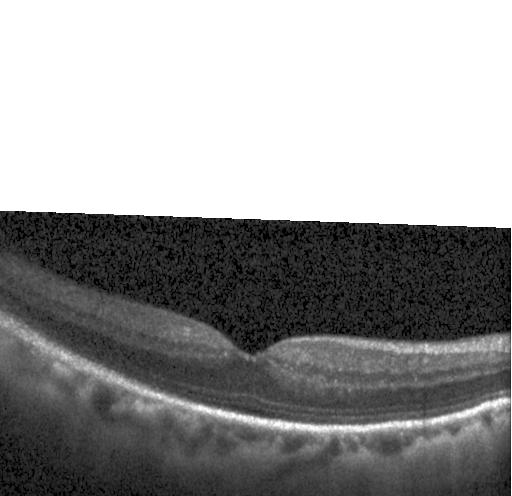

OCT finding: no CNV, no DME, and no drusen.